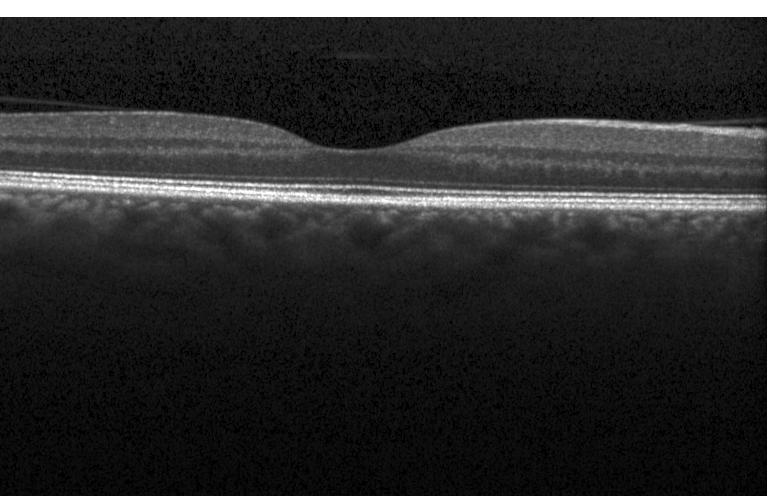
Macular OCT: neither CNV, DME, nor drusen.